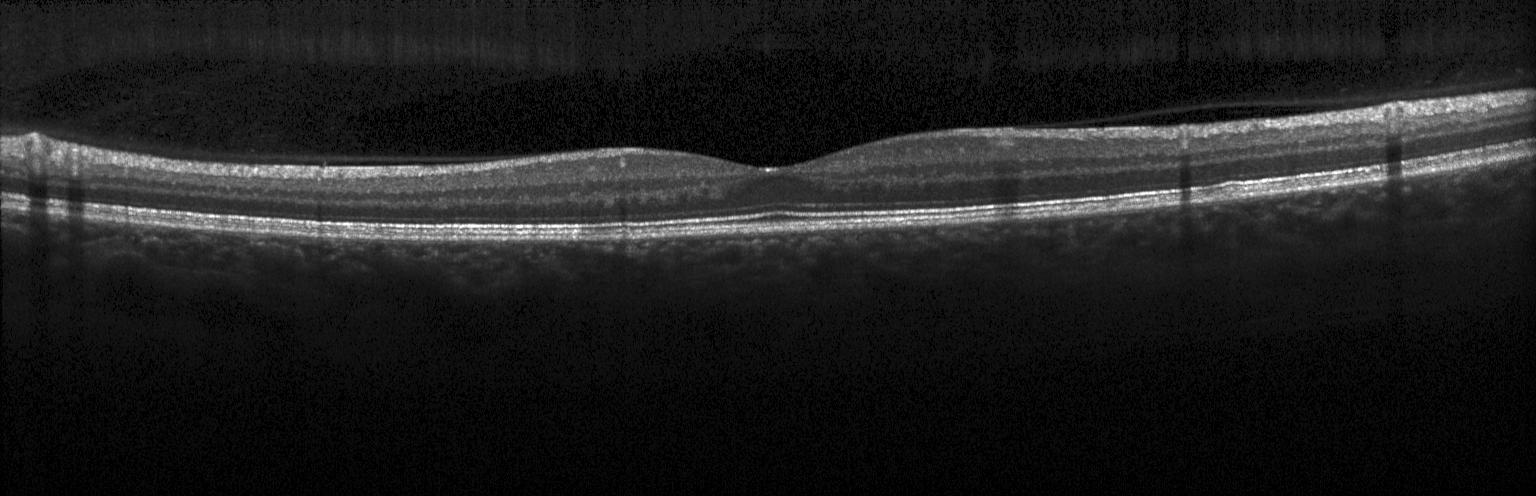
Assessment: no evidence of CNV, DME, or drusen.